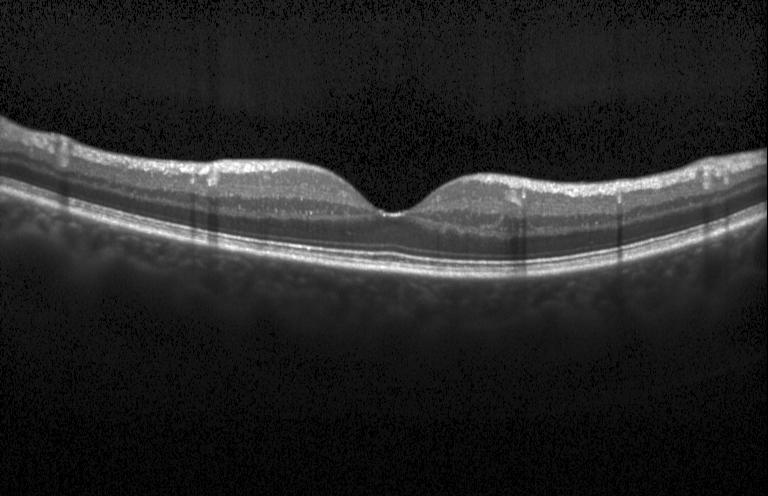

Retinal OCT cross-section
Finding: no choroidal neovascularization, no diabetic macular edema, and no drusen.